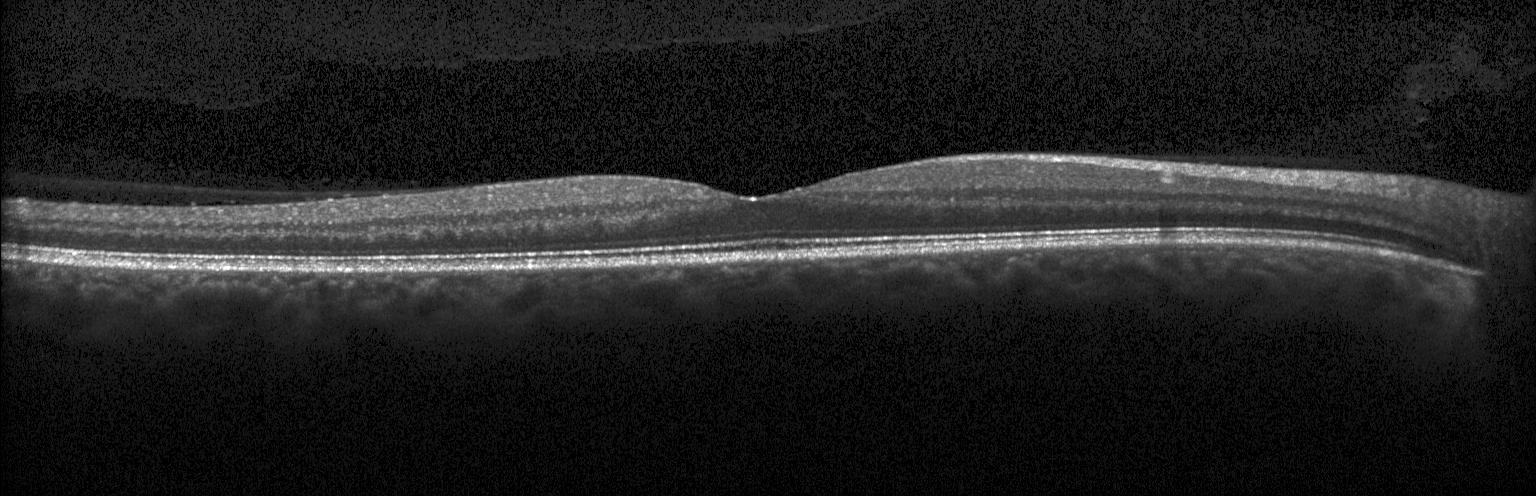 OCT scan showing neither choroidal neovascularization, diabetic macular edema, nor drusen.